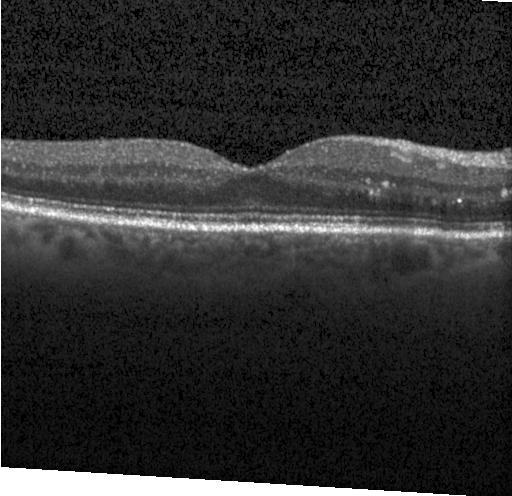
Retinal OCT cross-section. Assessment: neither choroidal neovascularization, diabetic macular edema, nor drusen.